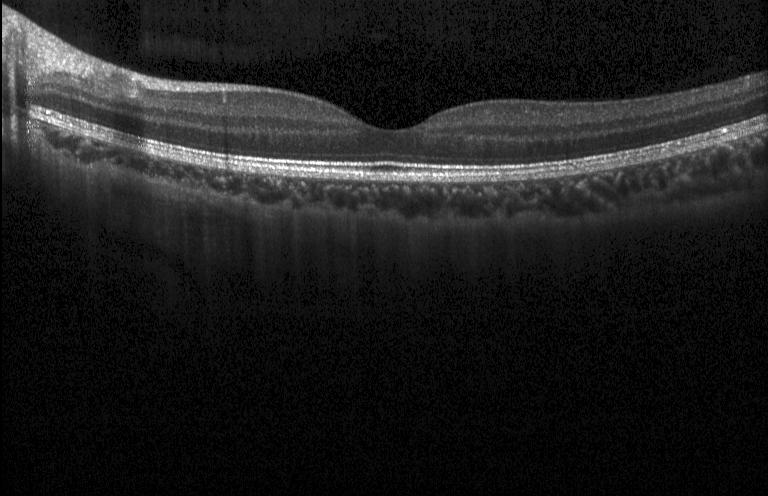
Heidelberg Spectralis. Spectral-domain OCT. Optical coherence tomography scan.
Diagnosis: no CNV, no DME, and no drusen.